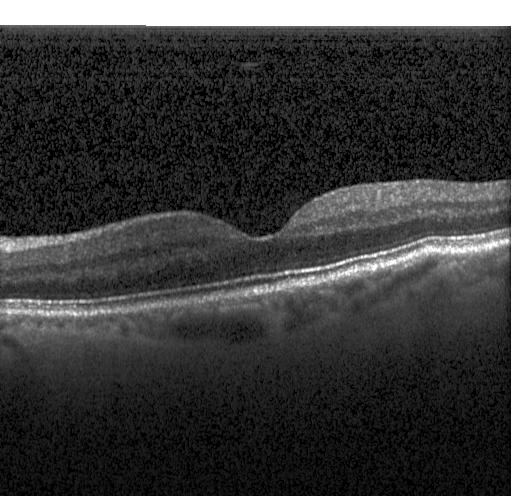 Horizontal scan through the fovea · retinal OCT cross-section · SD-OCT. The scan shows neither choroidal neovascularization, diabetic macular edema, nor drusen.